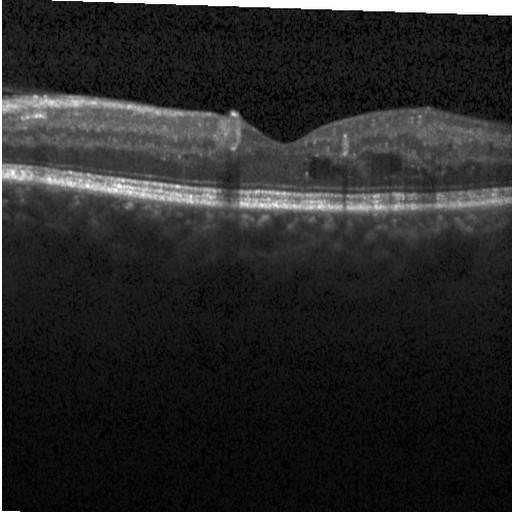
Finding: diabetic macular edema (DME).